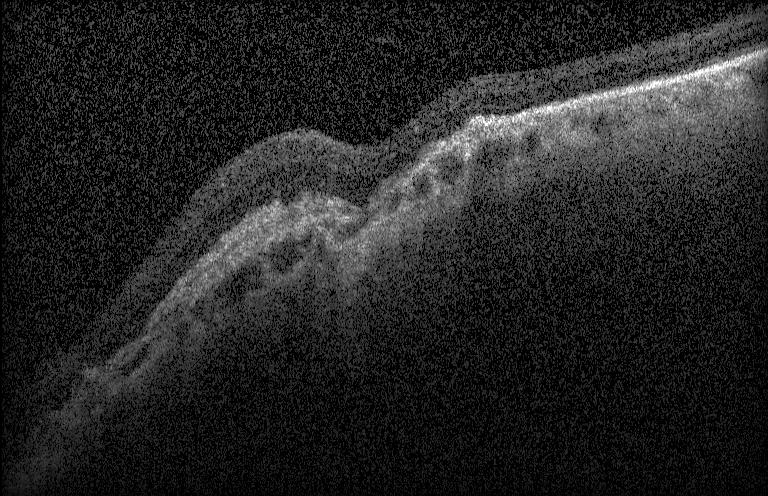 OCT line scan · centered on the fovea — A choroidal neovascular membrane.